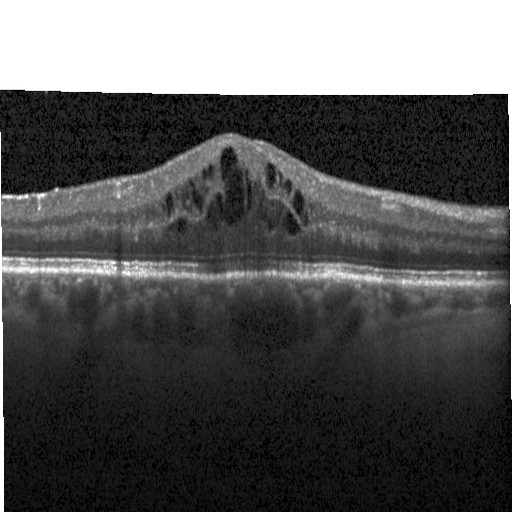

Diabetic macular edema.